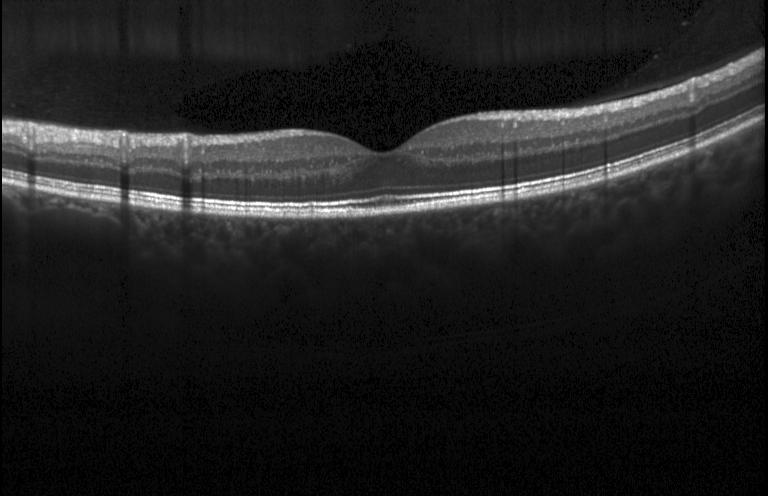

OCT line scan; horizontal scan through the fovea; acquired on a Heidelberg Spectralis — Dx: no CNV, no DME, and no drusen.